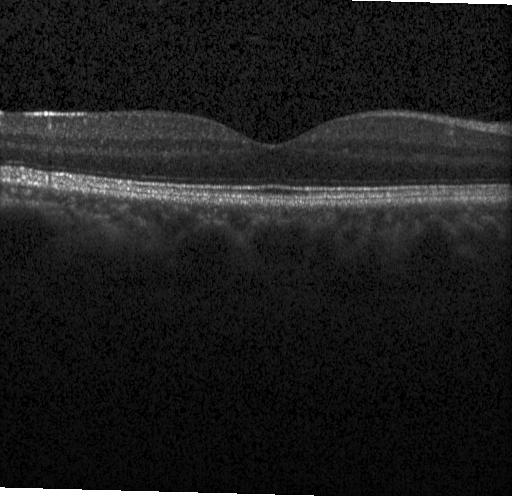
Retinal OCT cross-section showing neither choroidal neovascularization, diabetic macular edema, nor drusen.